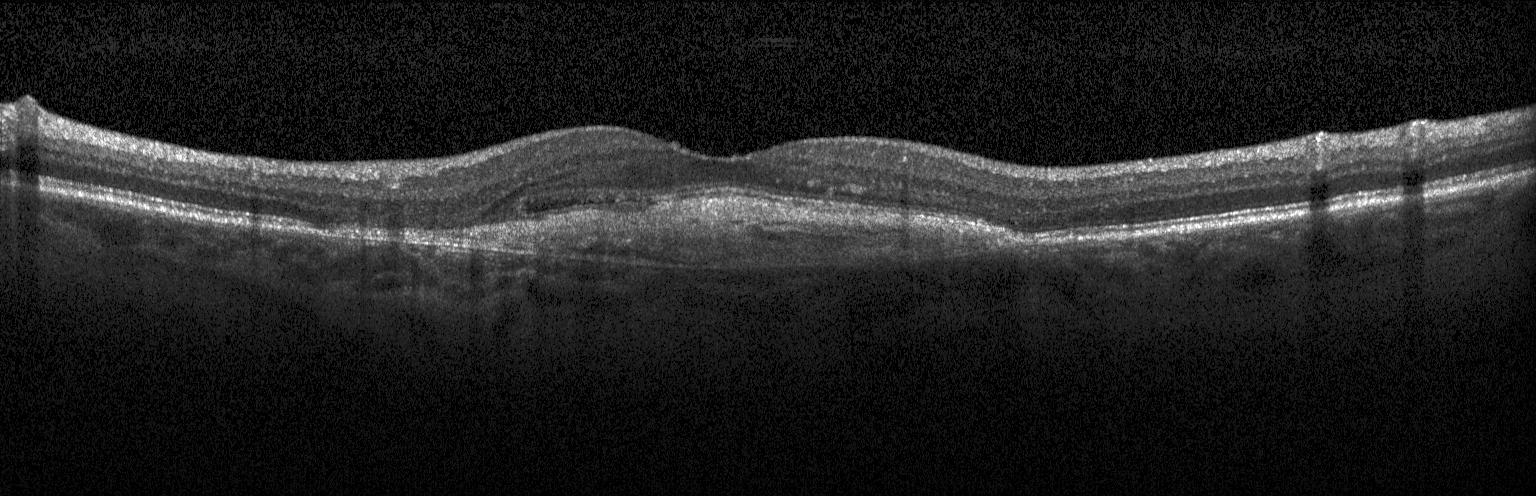
Retinal OCT cross-section; instrument: Heidelberg Spectralis — Diagnosis: choroidal neovascularization.